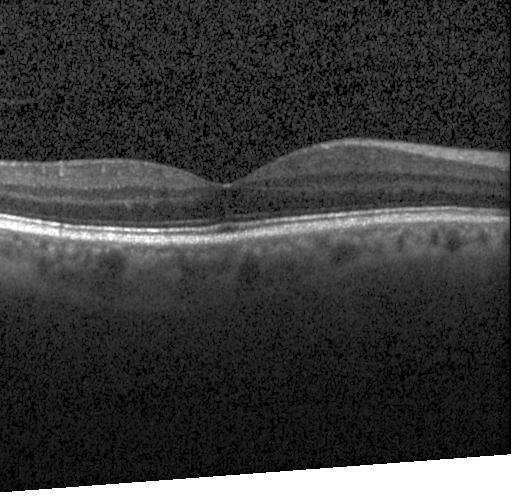

Impression: no choroidal neovascularization, no diabetic macular edema, and no drusen.